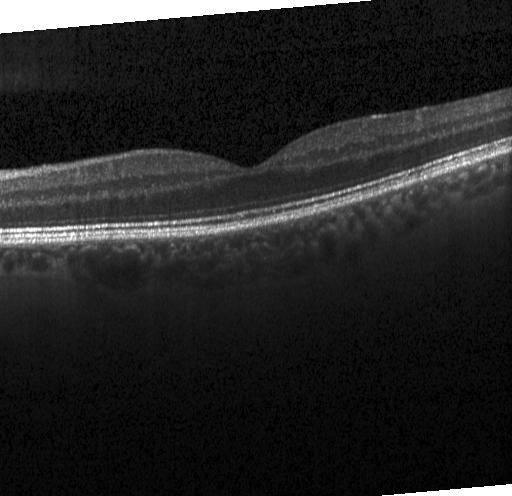 Finding: no evidence of choroidal neovascularization, diabetic macular edema, or drusen.